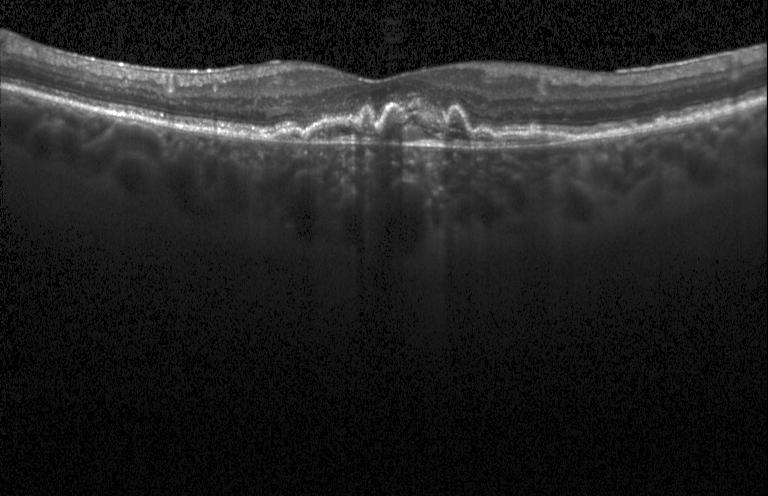

CNV.